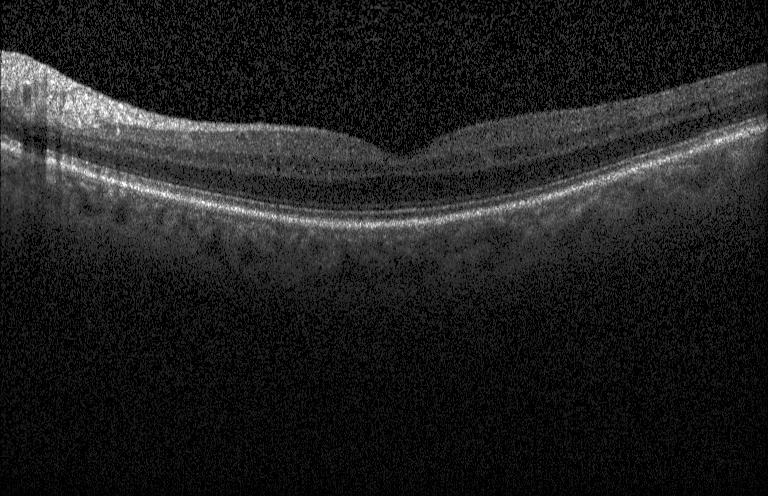

Optical coherence tomography B-scan. Through the macula. Spectral-domain optical coherence tomography. Acquired on a Heidelberg Spectralis — Impression: no choroidal neovascularization, no diabetic macular edema, and no drusen.